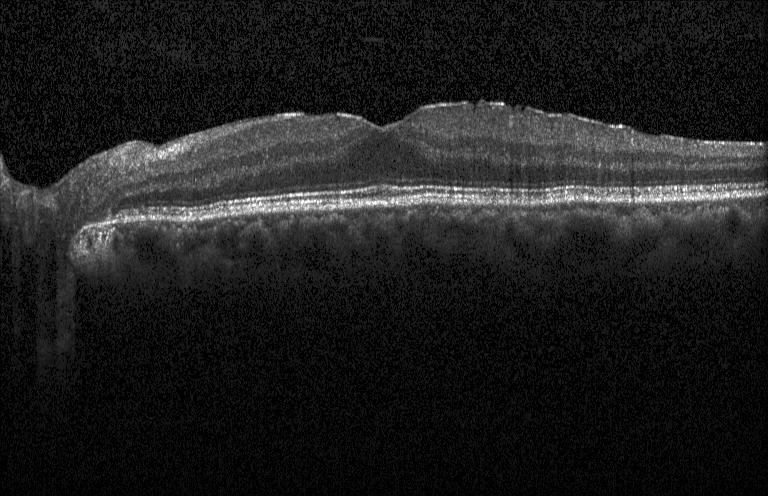
Optical coherence tomography scan. Assessment: neither CNV, DME, nor drusen.